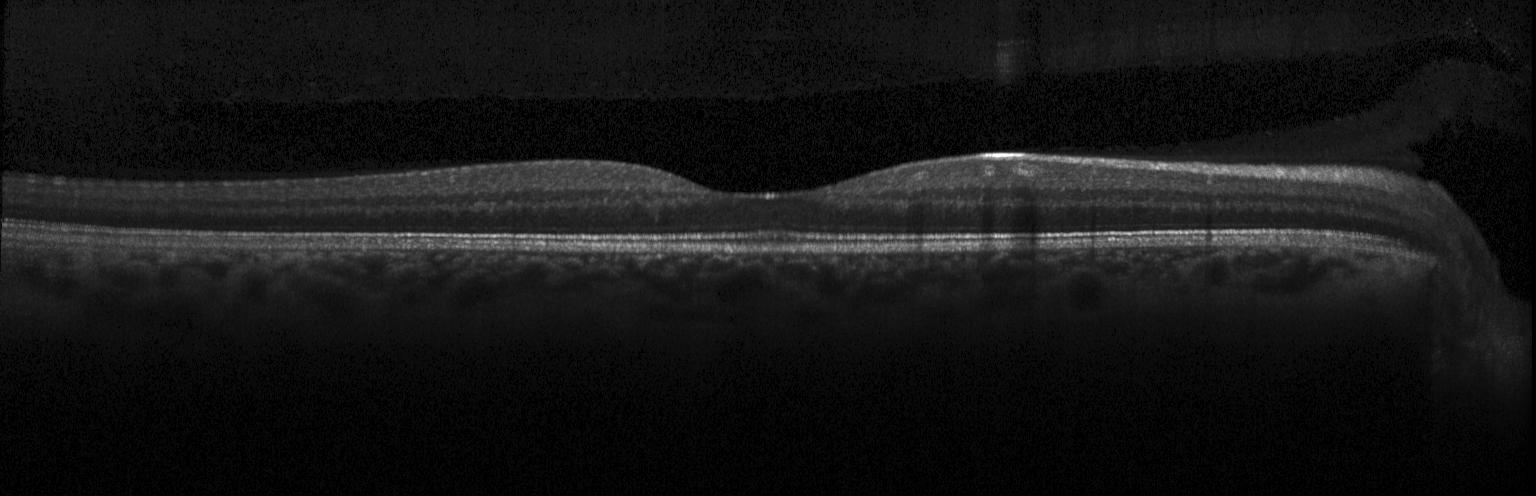
Impression: no evidence of choroidal neovascularization, diabetic macular edema, or drusen.